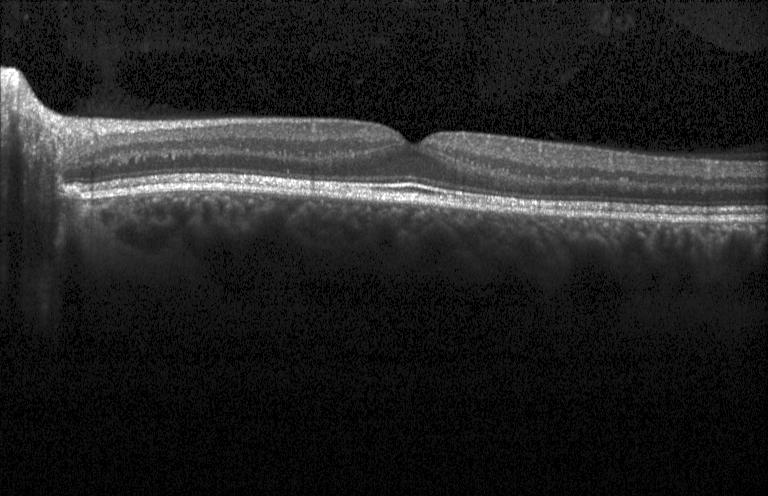
Fovea-centered; spectral-domain optical coherence tomography; Heidelberg Spectralis OCT system; optical coherence tomography B-scan.
Macular OCT: no CNV, DME, or drusen.